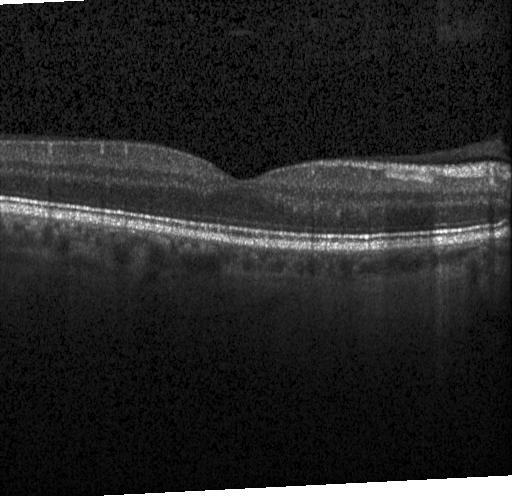

Retinal OCT B-scan.
This B-scan demonstrates no evidence of CNV, DME, or drusen.